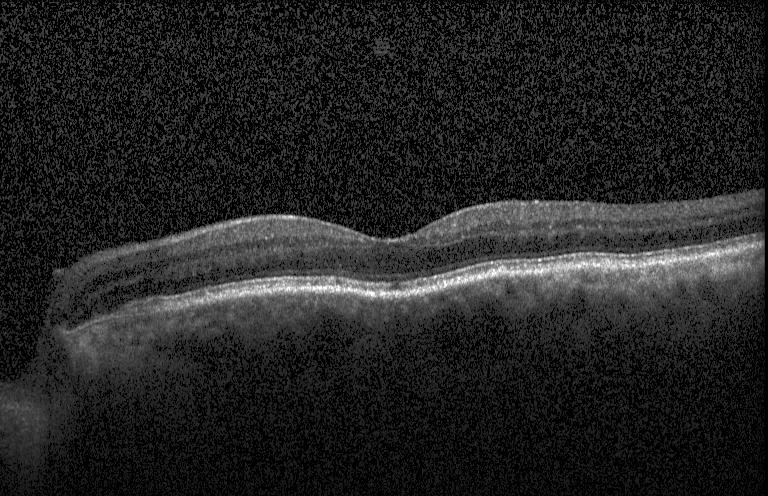 Impression: no evidence of choroidal neovascularization, diabetic macular edema, or drusen.